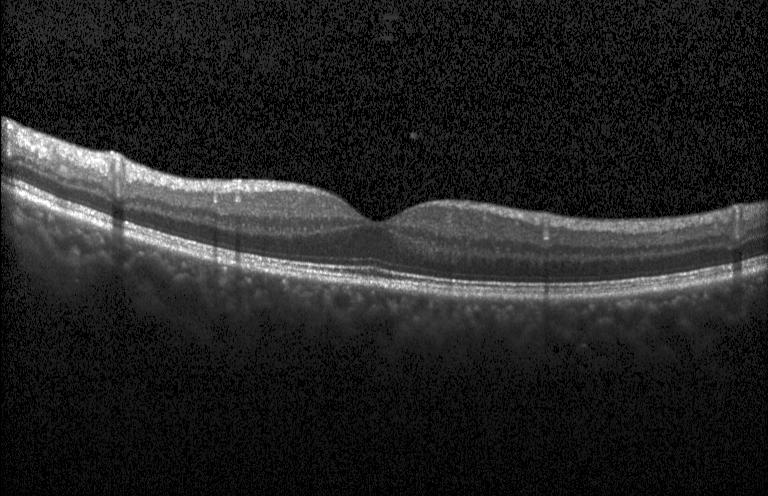

OCT finding: no choroidal neovascularization, no diabetic macular edema, and no drusen.